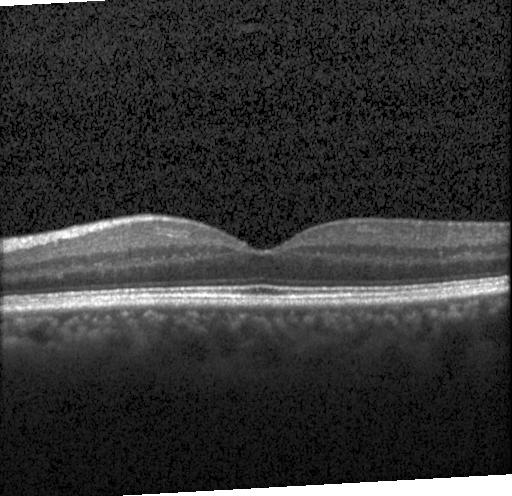
Heidelberg Spectralis OCT system; OCT line scan; macular scan
Diagnosis: no CNV, no DME, and no drusen.